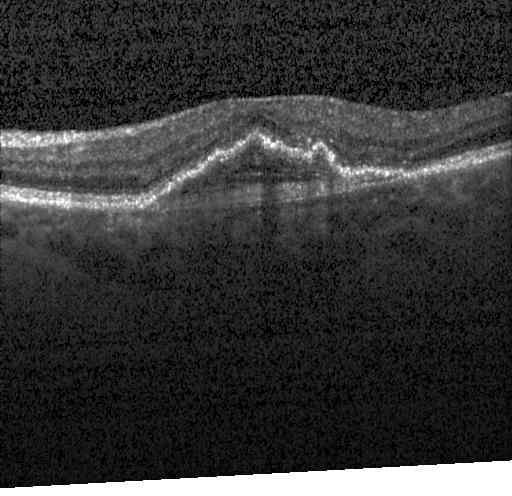 Spectral-domain OCT B-scan: CNV.